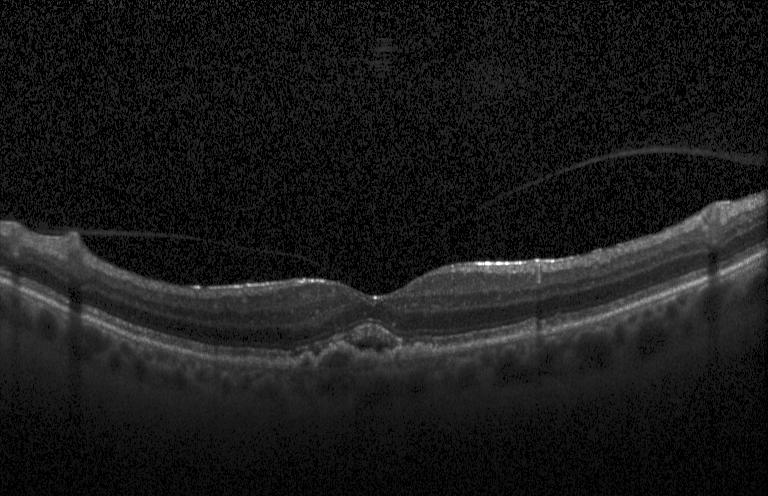 Optical coherence tomography scan; acquired on a Heidelberg Spectralis.
Impression: a choroidal neovascular membrane.